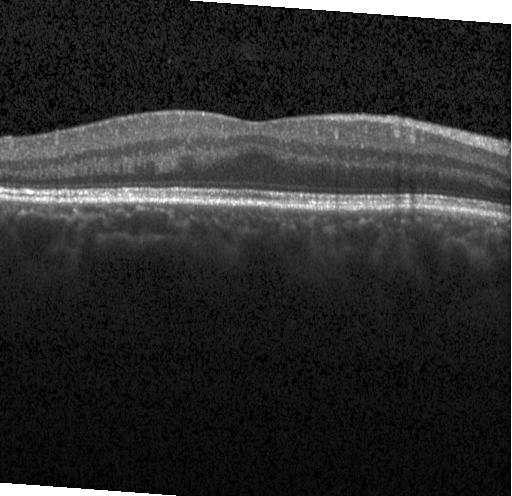

Optical coherence tomography B-scan; SD-OCT. OCT finding: no choroidal neovascularization, no diabetic macular edema, and no drusen.